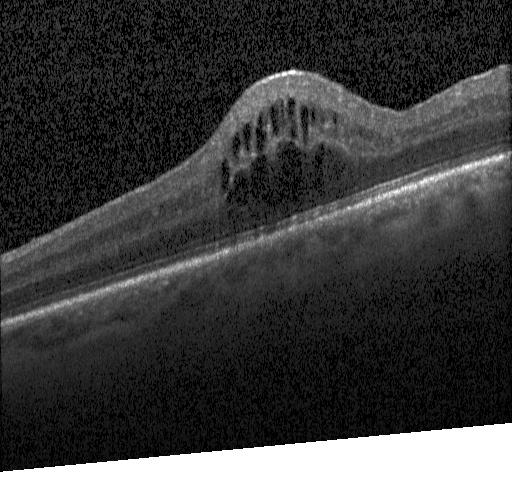 OCT finding: diabetic macular edema.